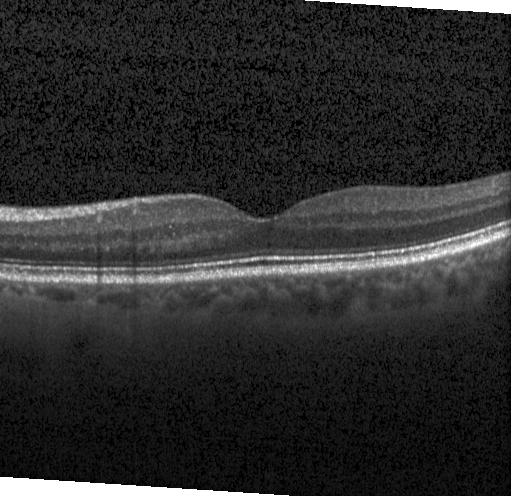 Optical coherence tomography B-scan, Heidelberg Spectralis. Diagnosis: neither choroidal neovascularization, diabetic macular edema, nor drusen.